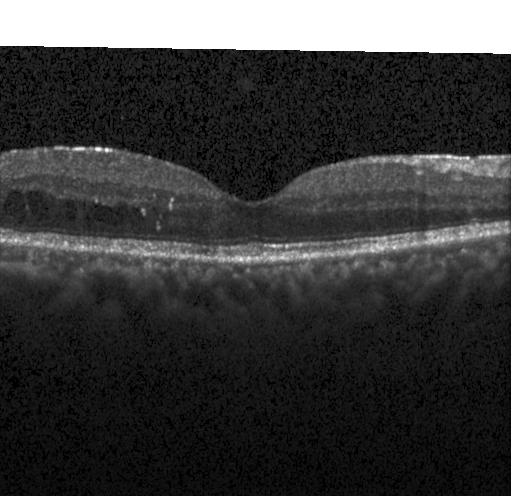 Spectral-domain OCT B-scan: diabetic macular edema (DME).